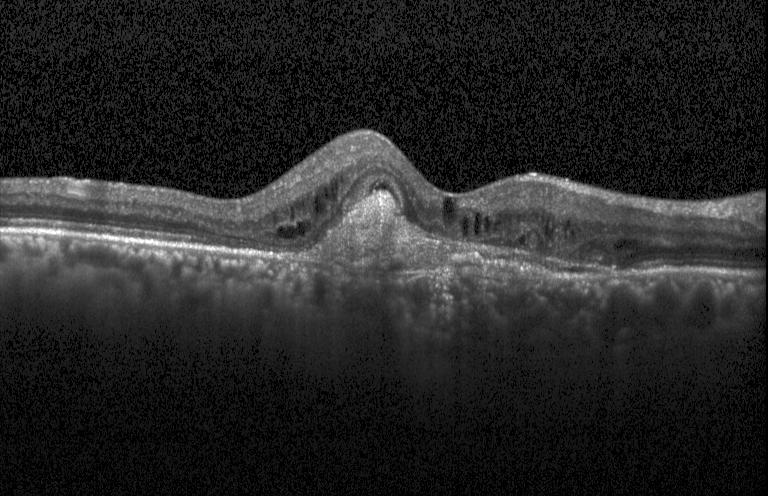
Centered on the fovea · OCT B-scan.
Diagnosis: a choroidal neovascular membrane.